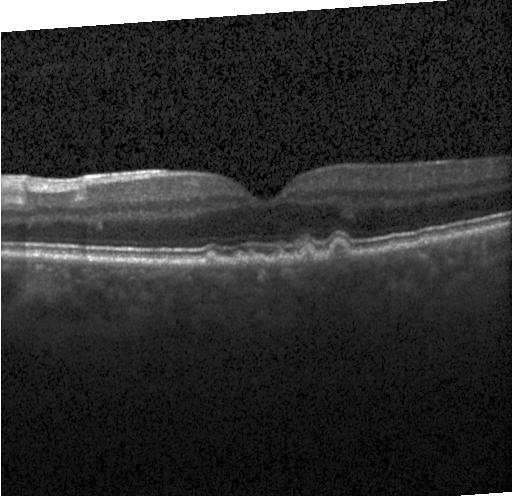
Optical coherence tomography B-scan.
Impression: drusen.